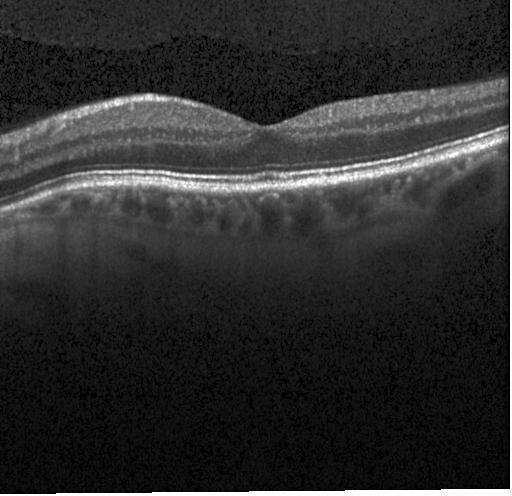
OCT B-scan showing no choroidal neovascularization, no diabetic macular edema, and no drusen.